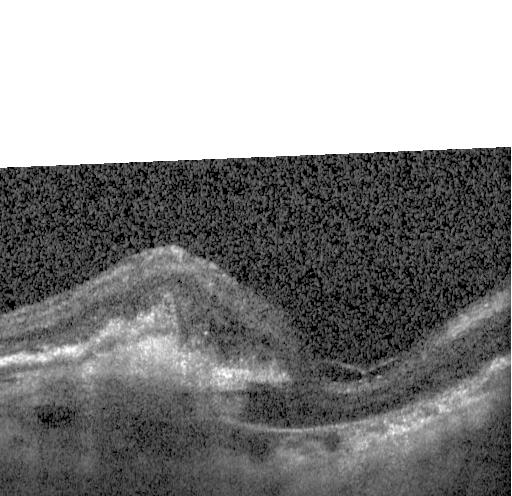

Optical coherence tomography B-scan.
This B-scan demonstrates a choroidal neovascular membrane.